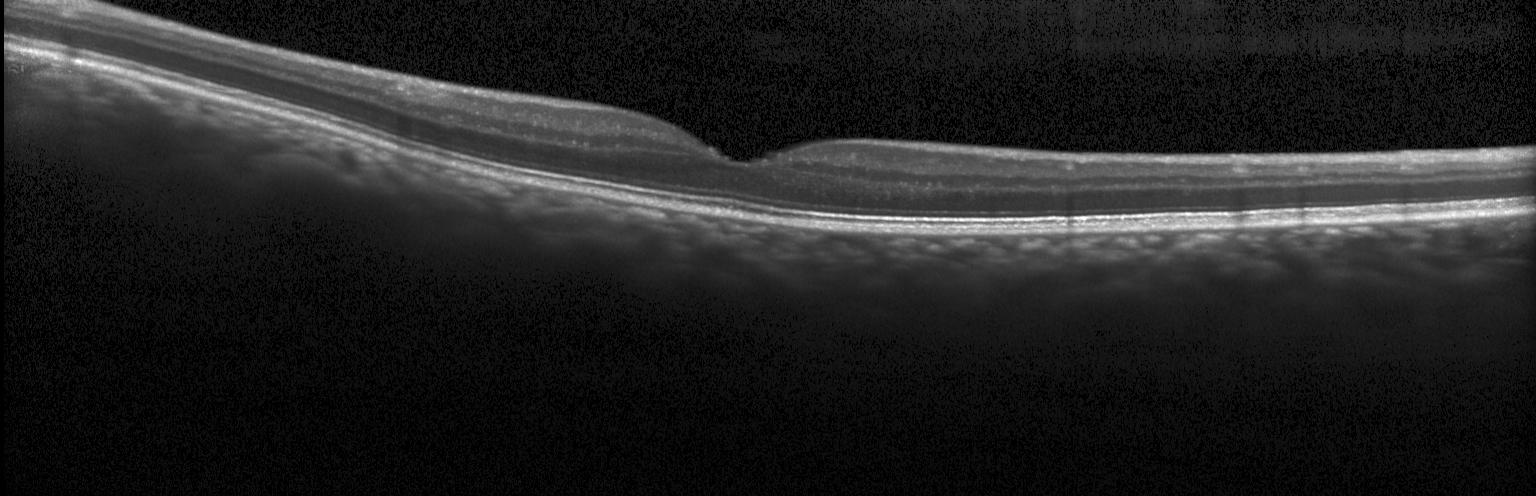
Optical coherence tomography scan.
Finding: no CNV, DME, or drusen.